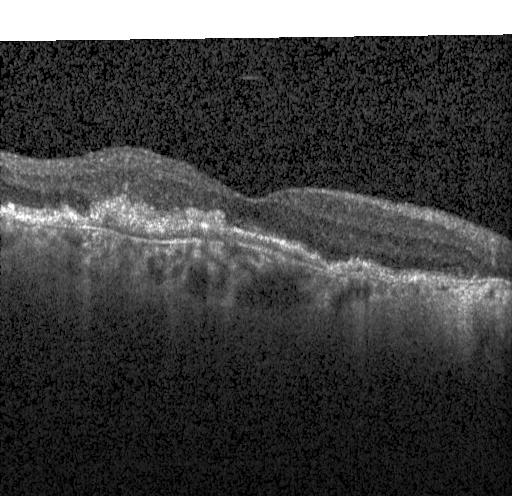

OCT B-scan. SD-OCT — Dx: a choroidal neovascular membrane.